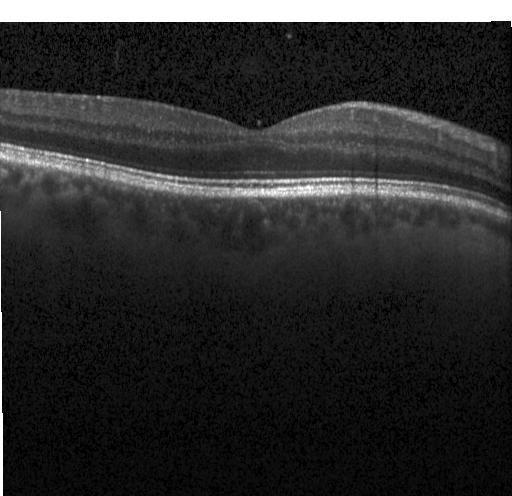
Assessment: no choroidal neovascularization, diabetic macular edema, or drusen.